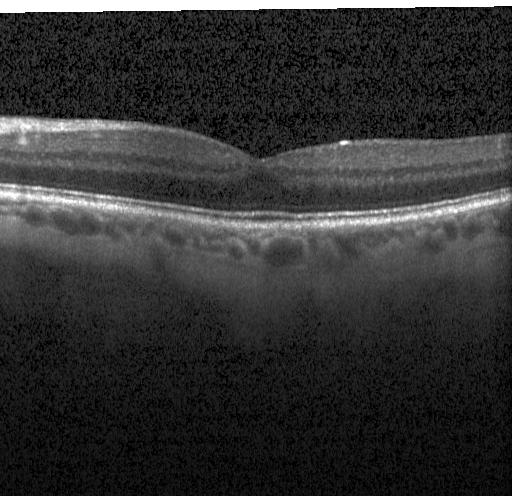
OCT line scan. OCT finding: no CNV, no DME, and no drusen.